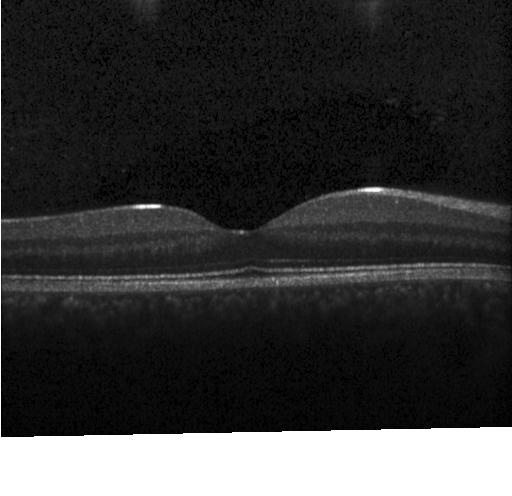
Spectral-domain OCT, retinal OCT B-scan, acquired on a Heidelberg Spectralis
The scan shows no choroidal neovascularization, no diabetic macular edema, and no drusen.